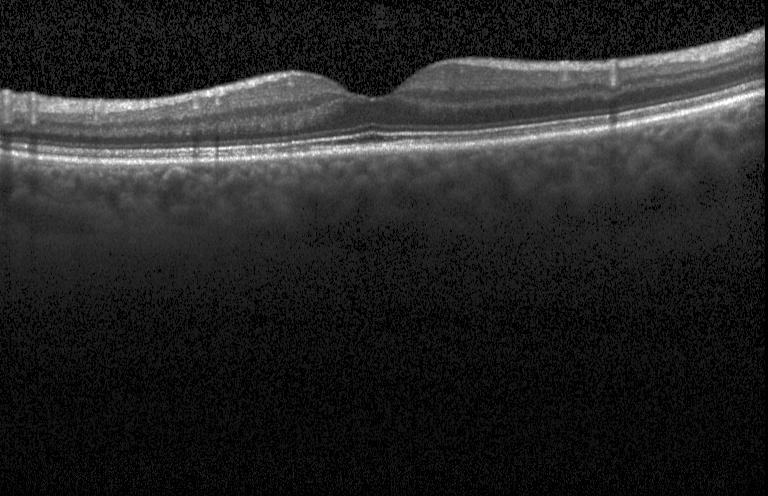
Retinal OCT B-scan · centered on the fovea.
This B-scan demonstrates no choroidal neovascularization, no diabetic macular edema, and no drusen.